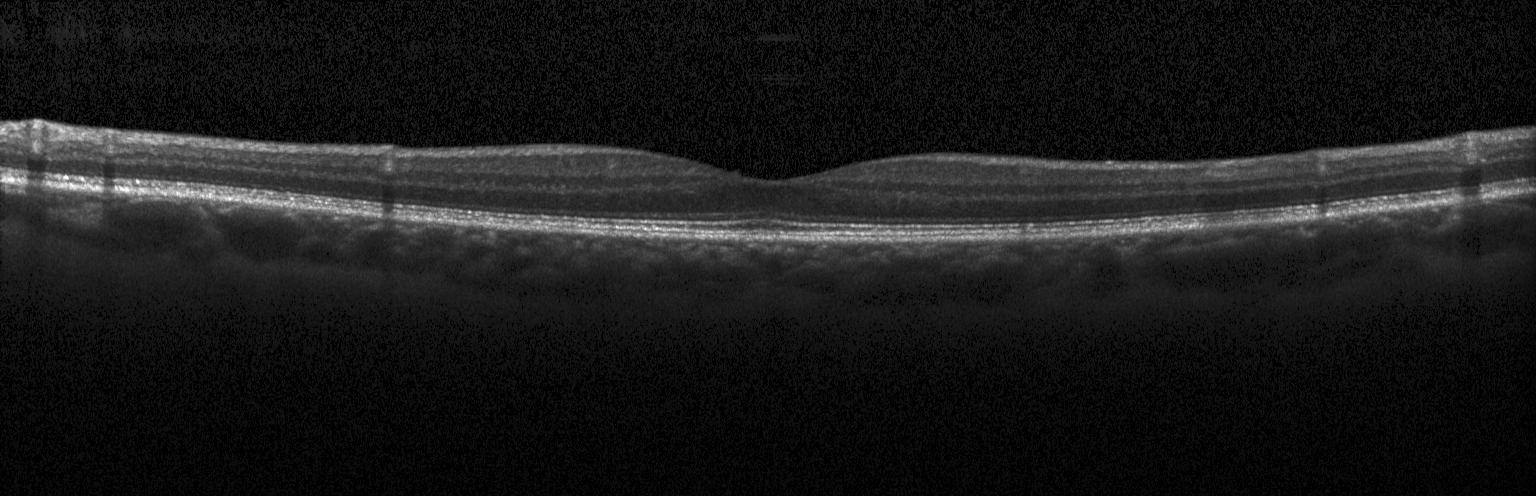

Optical coherence tomography B-scan
Macular OCT: no choroidal neovascularization, diabetic macular edema, or drusen.